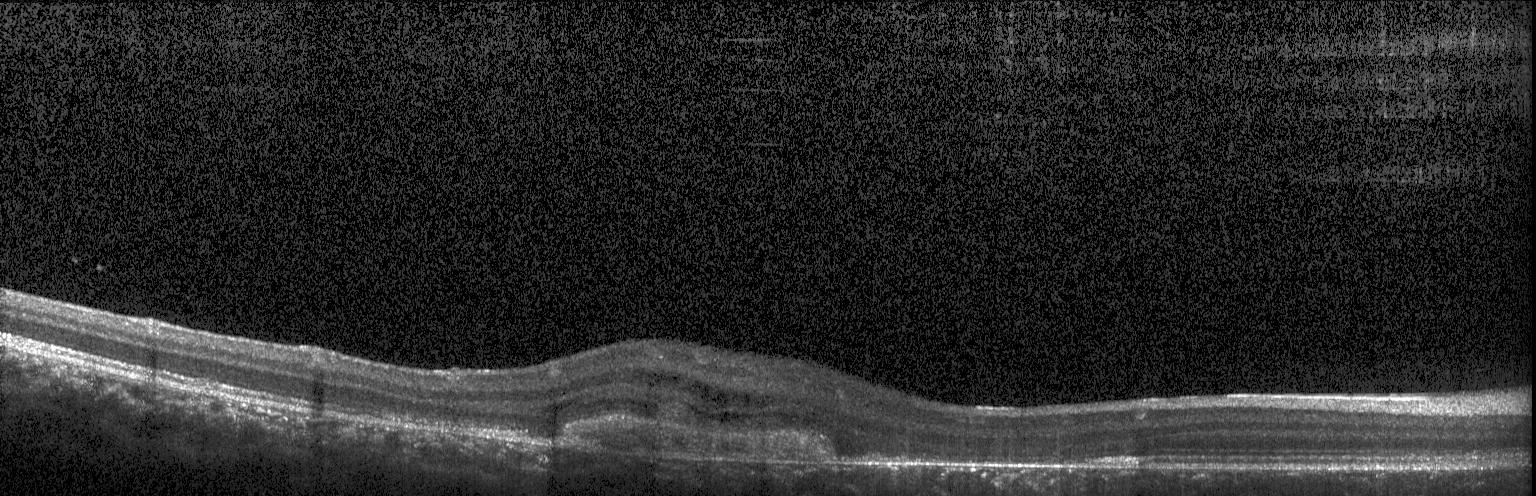

Heidelberg Spectralis OCT system, OCT B-scan, spectral-domain OCT.
This B-scan demonstrates a choroidal neovascular membrane.